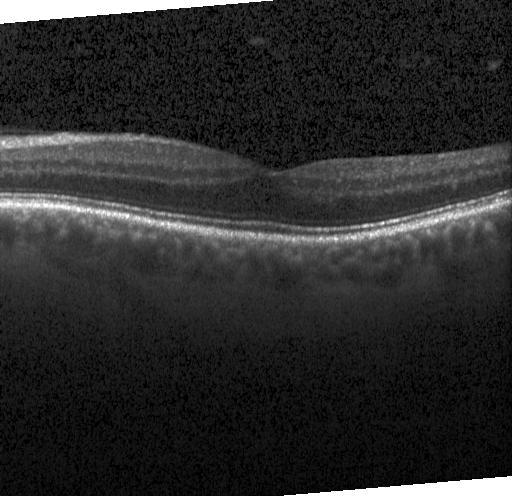 Retinal OCT B-scan
The scan shows neither choroidal neovascularization, diabetic macular edema, nor drusen.